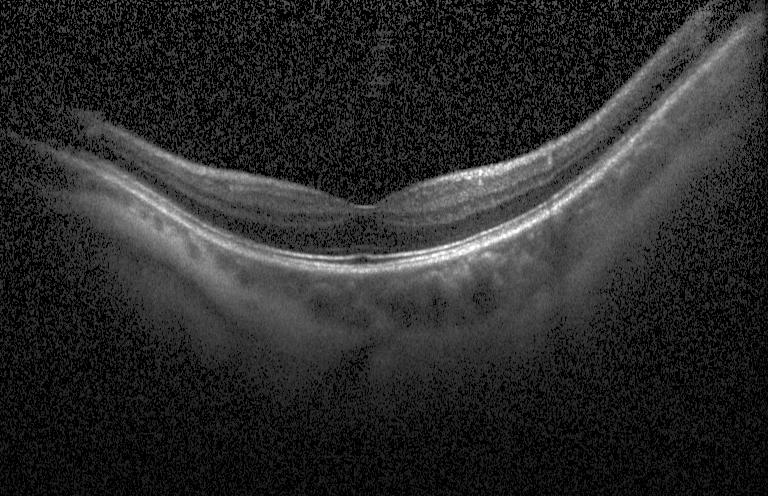

Optical coherence tomography B-scan · centered on the fovea · SD-OCT
No CNV, DME, or drusen.